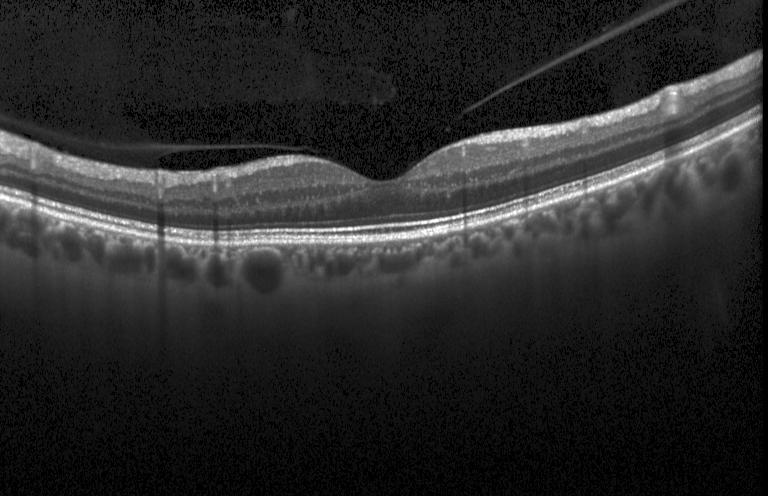
Heidelberg Spectralis OCT system · SD-OCT · centered on the fovea · optical coherence tomography scan. Diagnosis: no evidence of CNV, DME, or drusen.